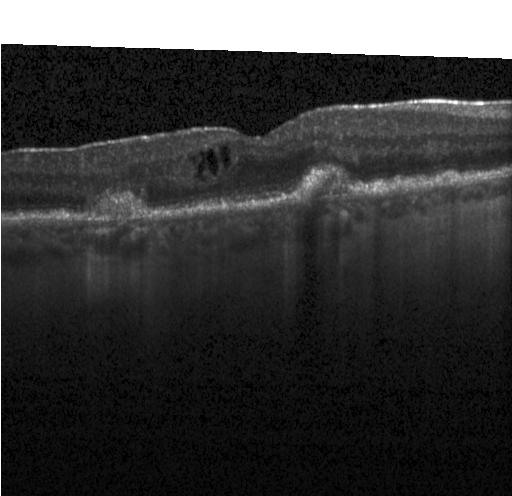
Retinal OCT B-scan. Impression: a choroidal neovascular membrane.